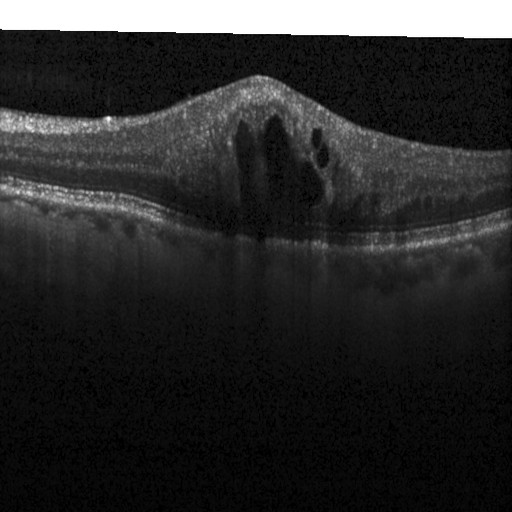

SD-OCT, OCT line scan, Heidelberg Spectralis — Assessment: diabetic macular edema.